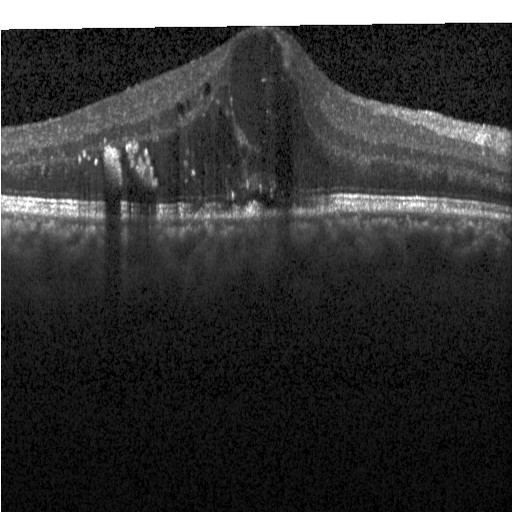
OCT B-scan · SD-OCT
Finding: DME.